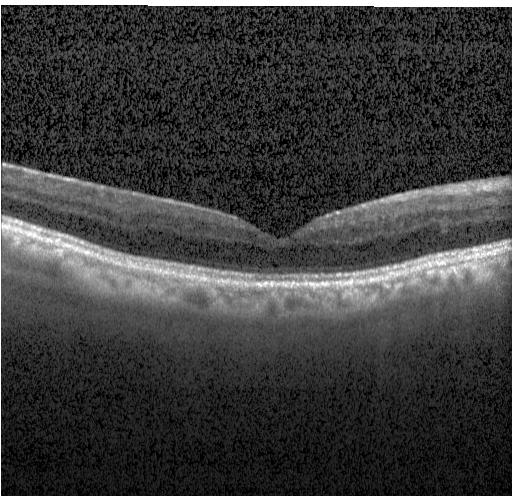
Retinal OCT cross-section — Assessment: no choroidal neovascularization, no diabetic macular edema, and no drusen.